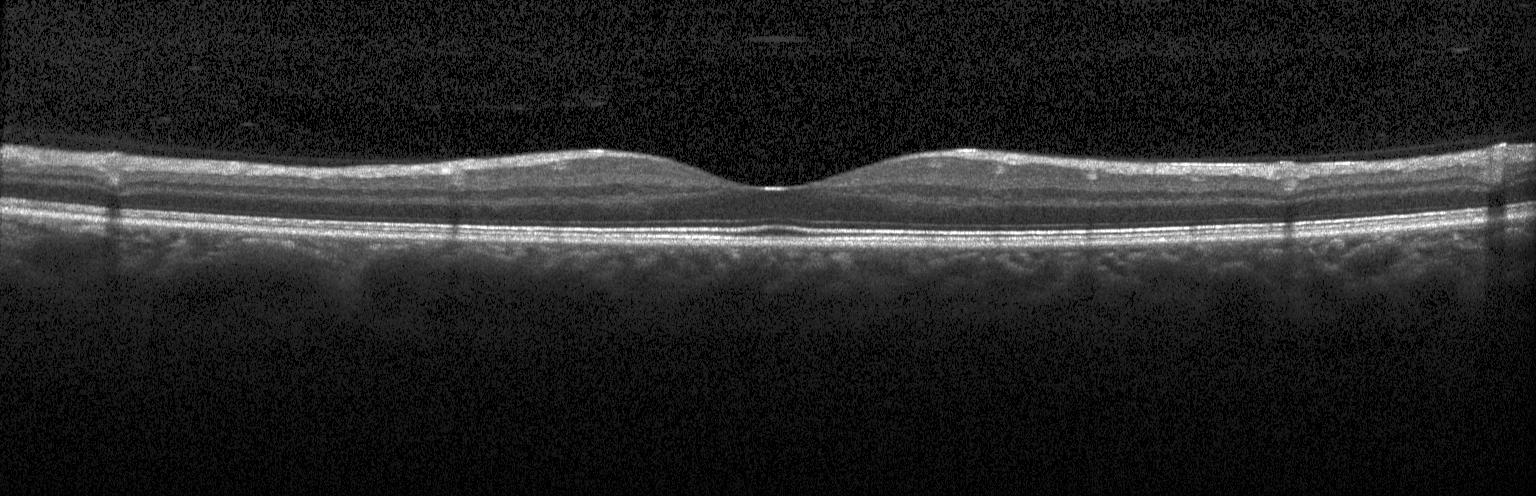

OCT line scan
Finding: no evidence of CNV, DME, or drusen.